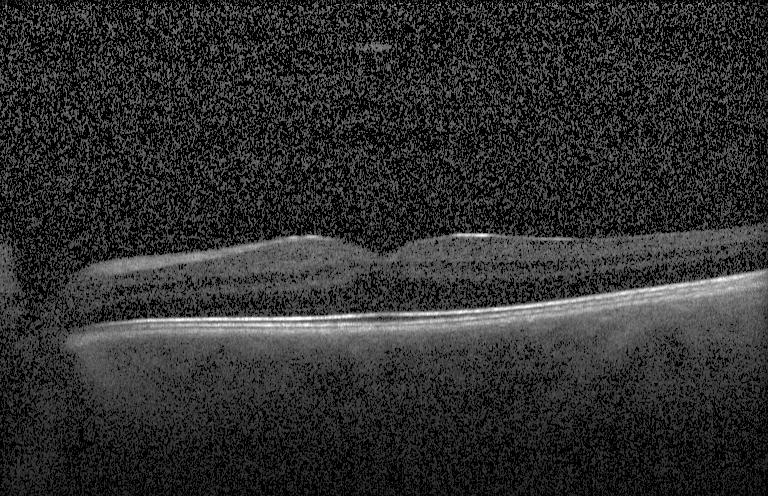

Optical coherence tomography scan, spectral-domain OCT, horizontal scan through the fovea — The scan shows no choroidal neovascularization, no diabetic macular edema, and no drusen.